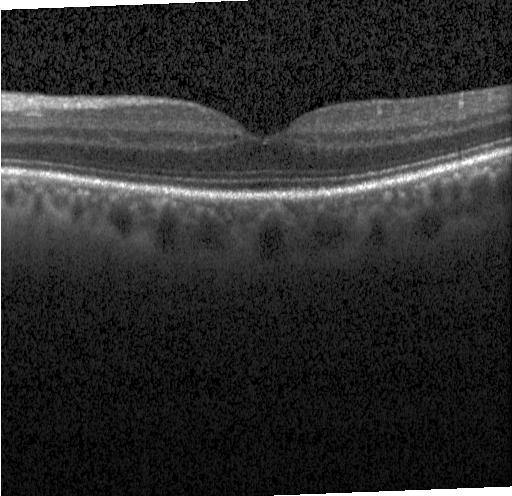 Heidelberg Spectralis OCT system · through the macula · spectral-domain OCT · retinal OCT B-scan — OCT finding: no evidence of choroidal neovascularization, diabetic macular edema, or drusen.